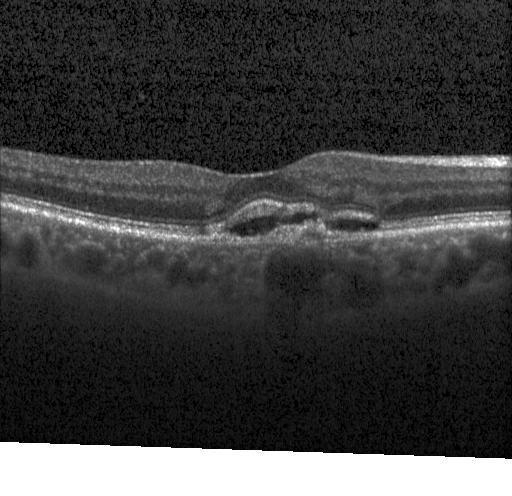

Macular scan · spectral-domain OCT · retinal OCT cross-section
This B-scan demonstrates CNV.